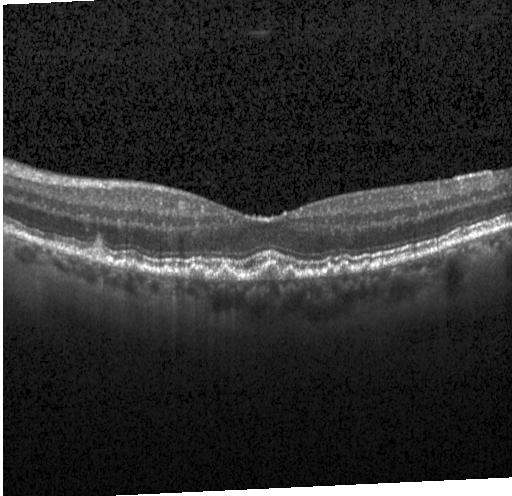 Diagnosis: multiple drusen.